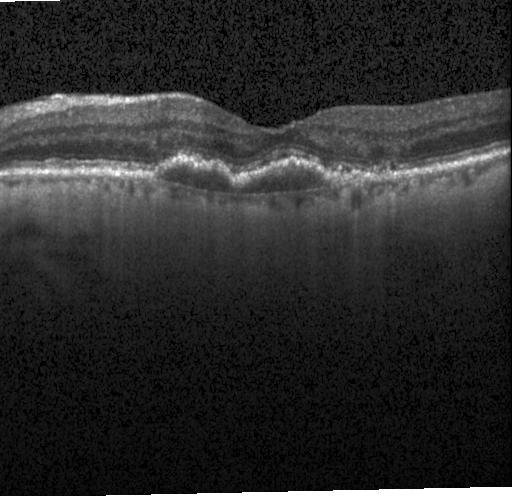
A choroidal neovascular membrane.